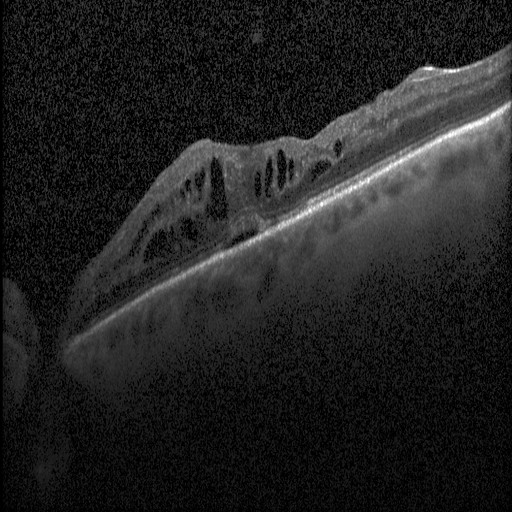 The scan shows diabetic macular edema (DME).